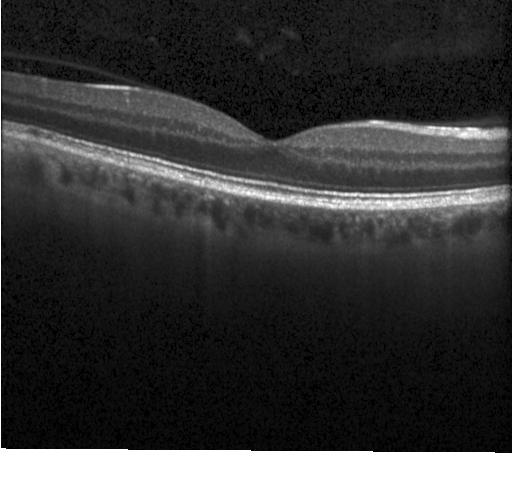 Spectral-domain OCT. Optical coherence tomography B-scan. Finding: neither choroidal neovascularization, diabetic macular edema, nor drusen.